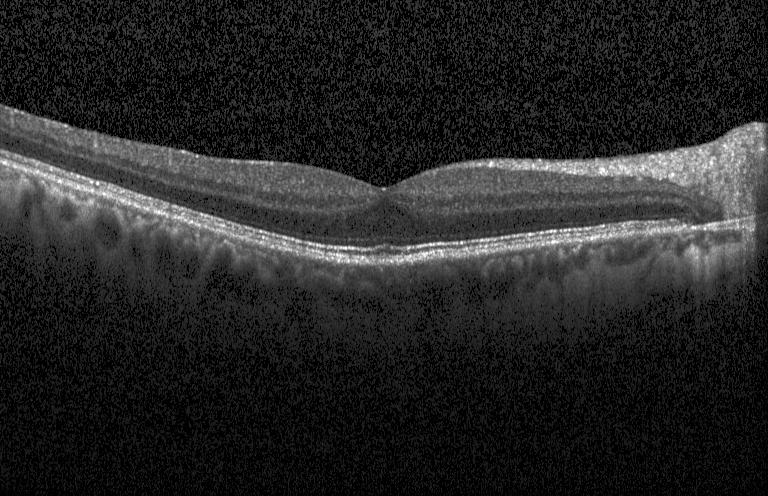 Optical coherence tomography B-scan, through the macula. Diagnosis: no evidence of choroidal neovascularization, diabetic macular edema, or drusen.